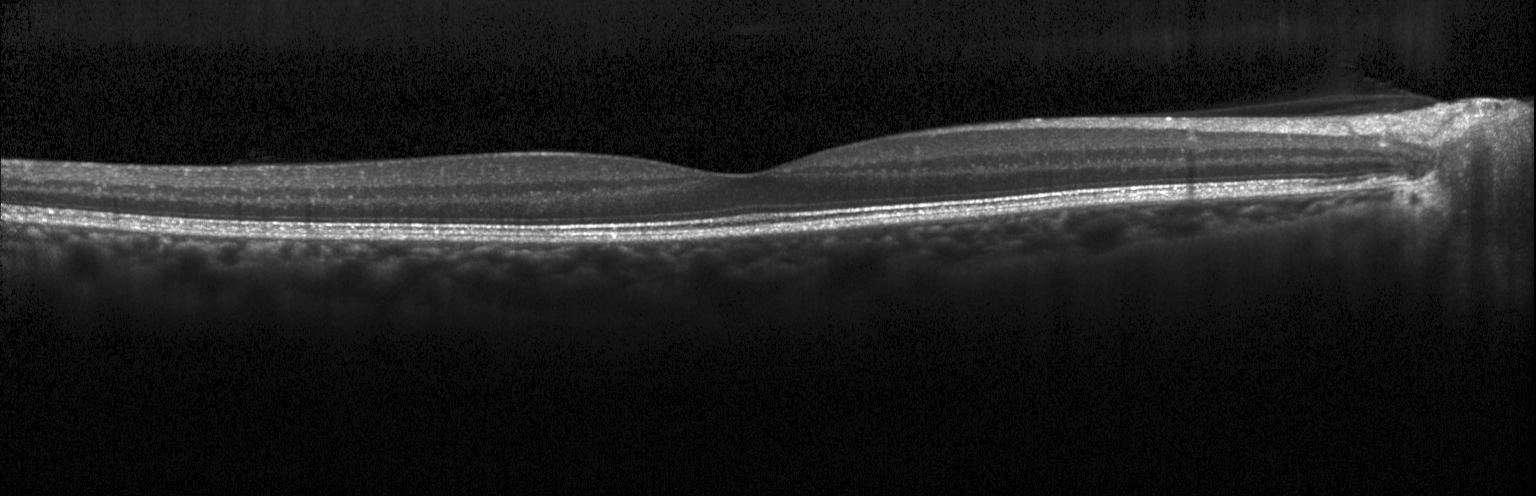
Heidelberg Spectralis · retinal OCT B-scan · centered on the fovea. Diagnosis: neither CNV, DME, nor drusen.